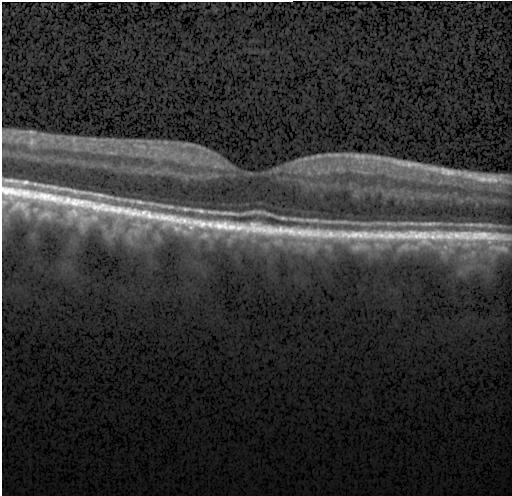
Through the macula. Retinal OCT B-scan
No evidence of choroidal neovascularization, diabetic macular edema, or drusen.